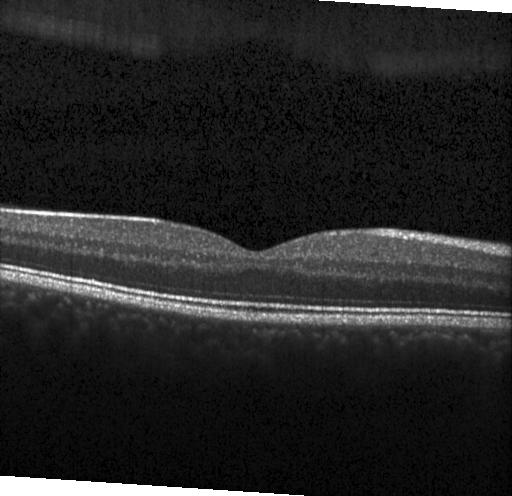 Diagnosis: no choroidal neovascularization, no diabetic macular edema, and no drusen.